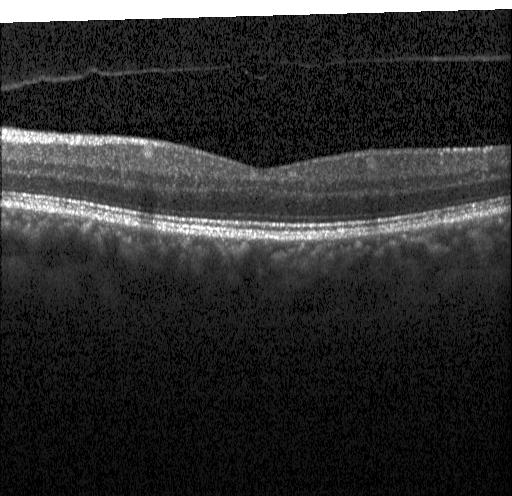 Retinal OCT B-scan. Heidelberg Spectralis OCT system
Impression: no choroidal neovascularization, no diabetic macular edema, and no drusen.